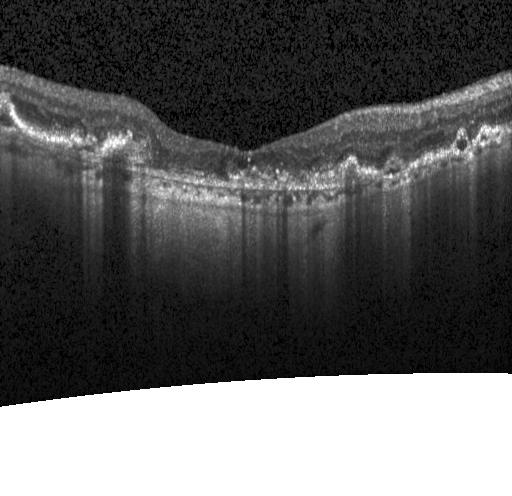
OCT line scan.
Impression: choroidal neovascularization (CNV).